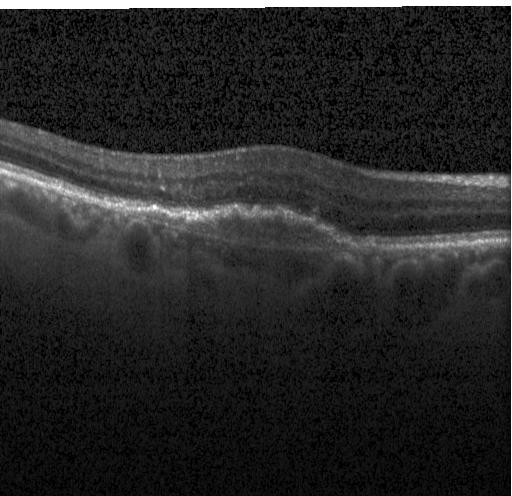

Heidelberg Spectralis · horizontal scan through the fovea · optical coherence tomography scan · spectral-domain optical coherence tomography. Impression: a choroidal neovascular membrane.